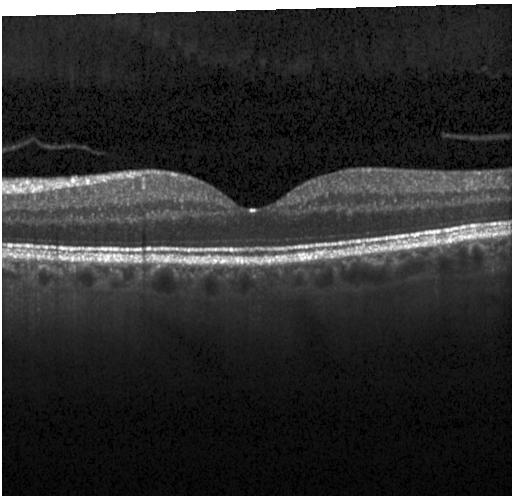

Retinal OCT cross-section; acquired on a Heidelberg Spectralis; through the macula. No evidence of choroidal neovascularization, diabetic macular edema, or drusen.